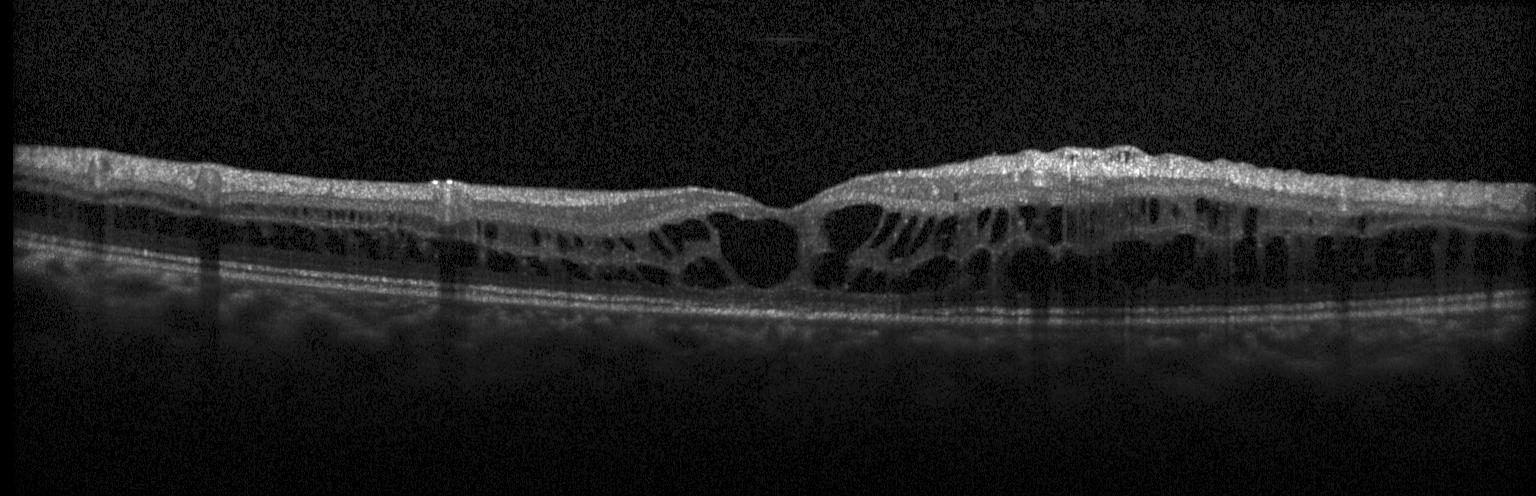

Diagnosis: diabetic macular edema.